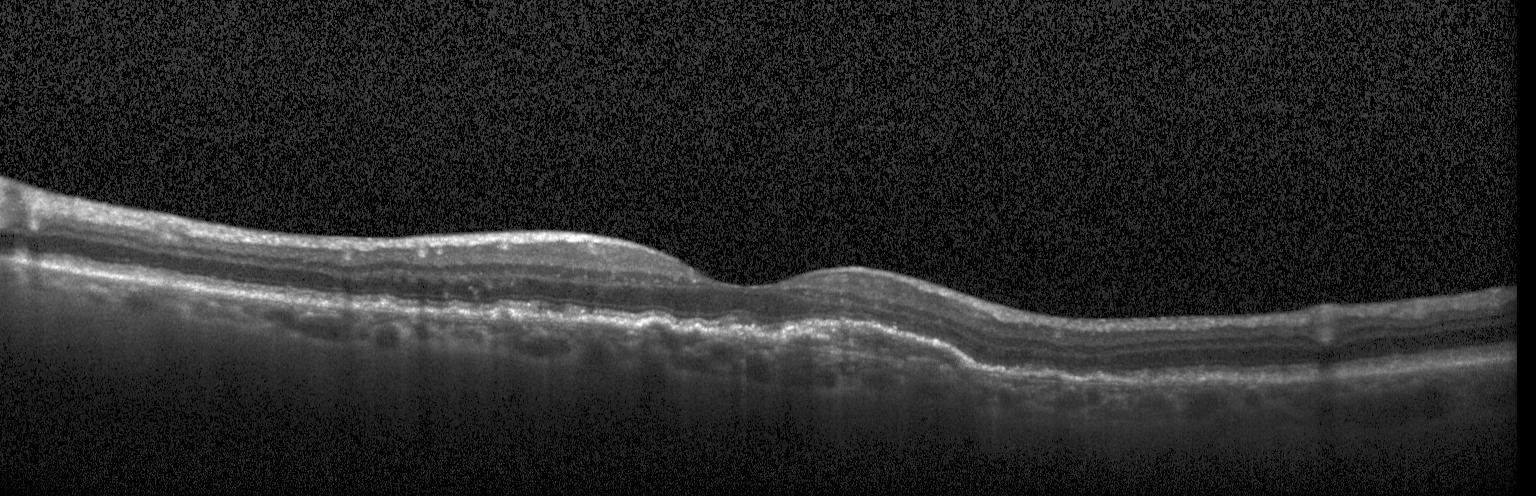 OCT scan showing CNV.